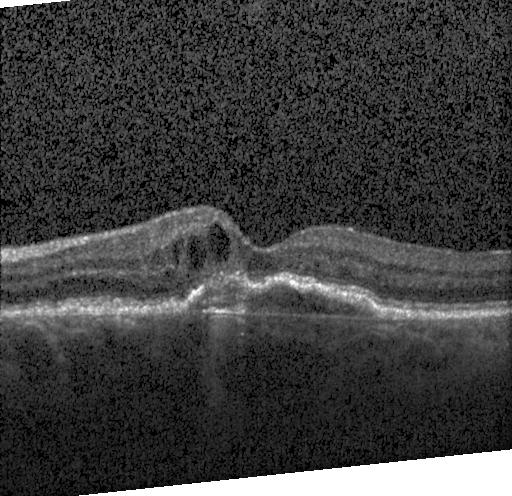

Spectral-domain OCT, instrument: Heidelberg Spectralis, optical coherence tomography scan
The scan shows CNV.